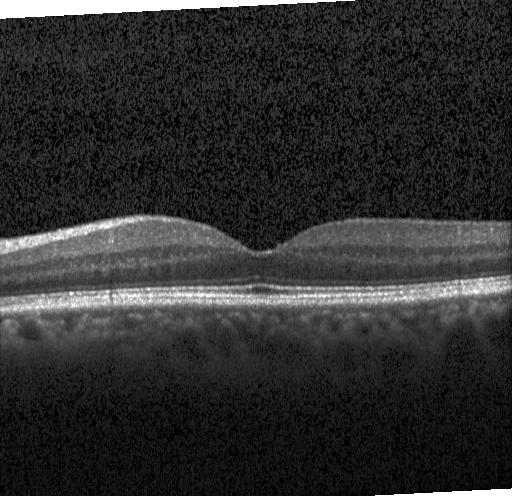 Retinal OCT cross-section showing no evidence of CNV, DME, or drusen.